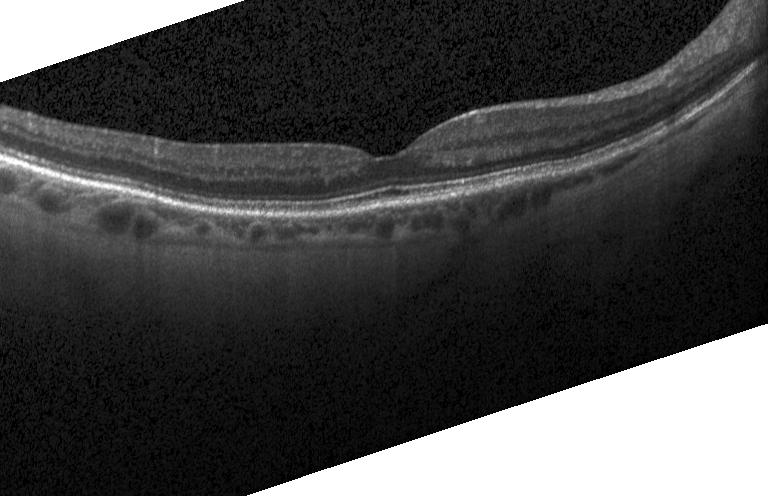
Spectral-domain OCT. Optical coherence tomography scan. Centered on the fovea
Impression: neither CNV, DME, nor drusen.